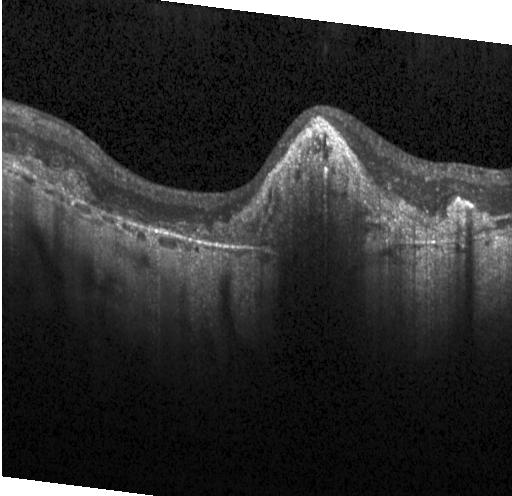
OCT B-scan · spectral-domain optical coherence tomography · macular scan · acquired on a Heidelberg Spectralis. Impression: CNV.